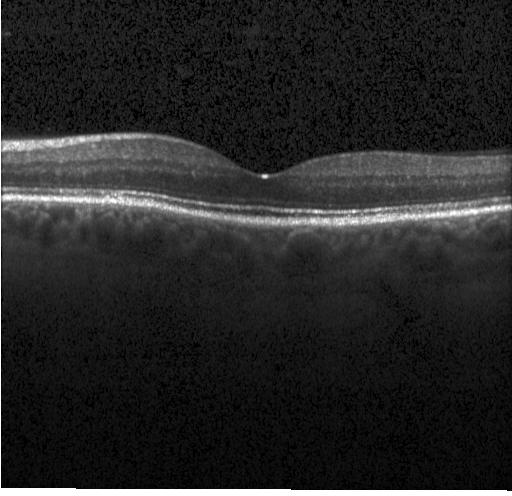
Retinal OCT B-scan. No choroidal neovascularization, no diabetic macular edema, and no drusen.